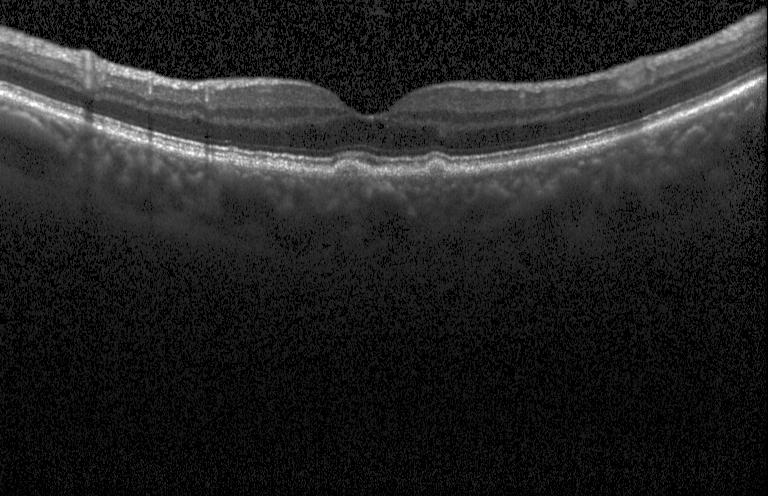

OCT line scan — Finding: sub-RPE drusenoid deposits.